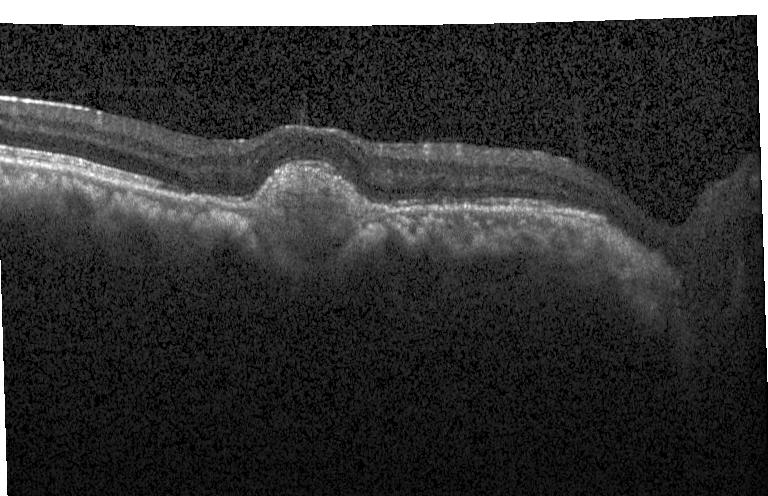 Optical coherence tomography B-scan, centered on the fovea — OCT finding: a choroidal neovascular membrane.